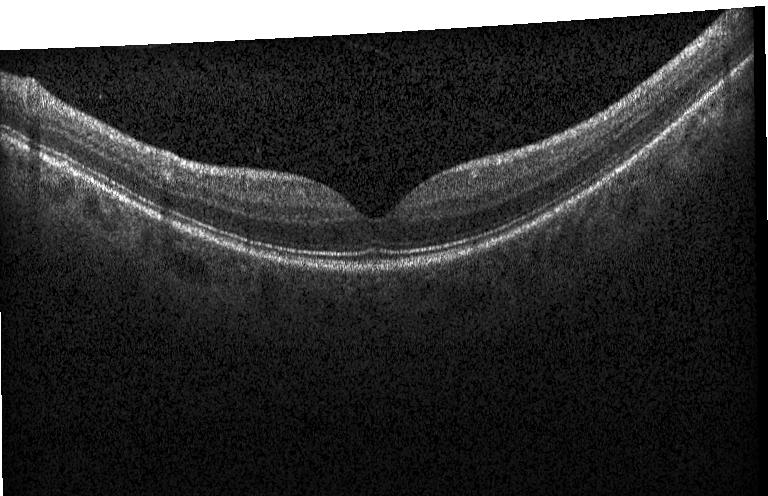

Macular scan; acquired on a Heidelberg Spectralis; spectral-domain OCT; optical coherence tomography B-scan
Finding: neither choroidal neovascularization, diabetic macular edema, nor drusen.